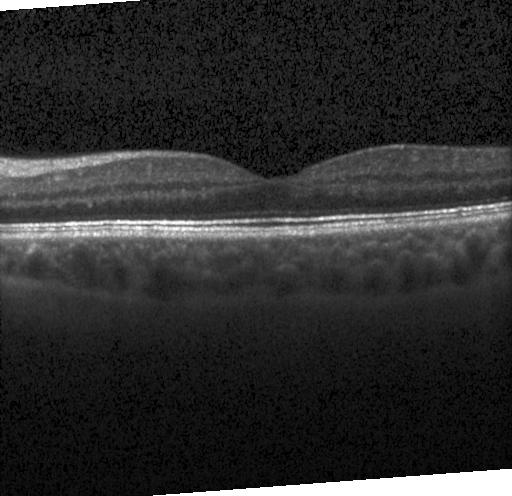 Spectral-domain OCT. Macular scan. Instrument: Heidelberg Spectralis. OCT line scan — Macular OCT: no evidence of choroidal neovascularization, diabetic macular edema, or drusen.